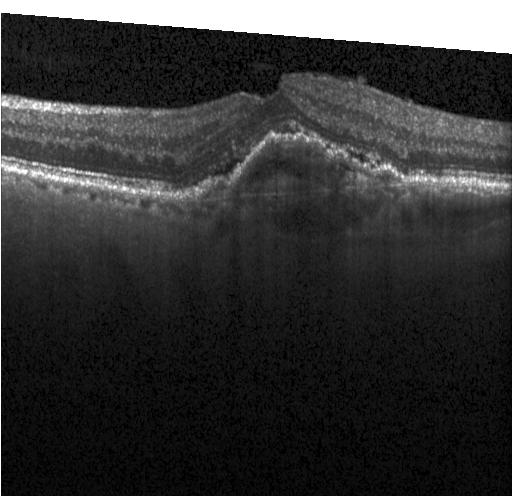
Through the macula; OCT B-scan; spectral-domain OCT
Finding: a choroidal neovascular membrane.